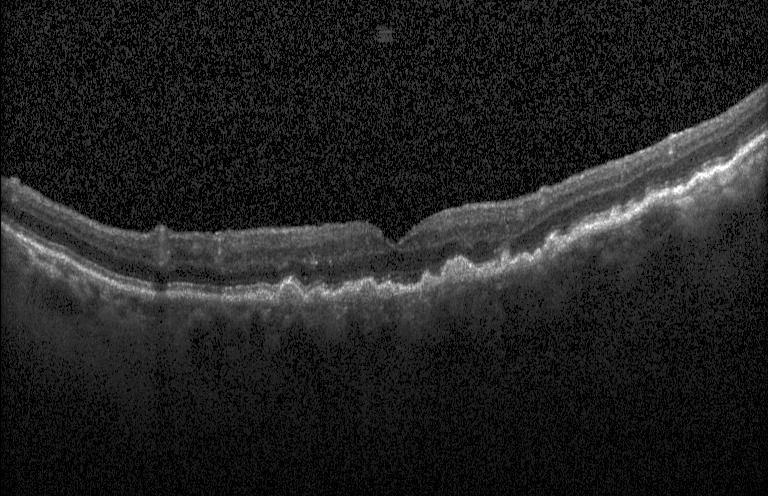

OCT line scan — Finding: sub-RPE drusenoid deposits.